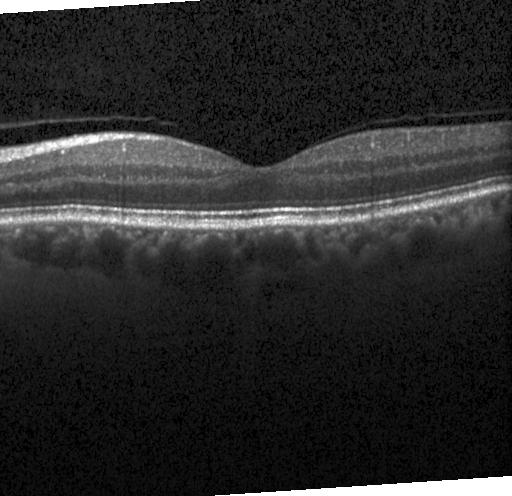
Macular scan. Retinal OCT B-scan. Acquired on a Heidelberg Spectralis. Spectral-domain OCT. Macular OCT: no choroidal neovascularization, no diabetic macular edema, and no drusen.